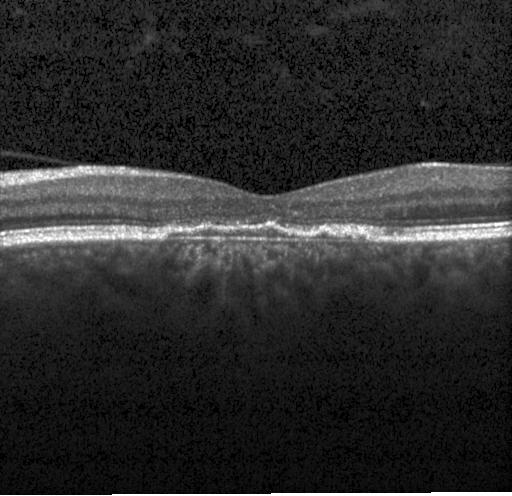 Acquired on a Heidelberg Spectralis, OCT B-scan, spectral-domain OCT. Macular OCT: a choroidal neovascular membrane.